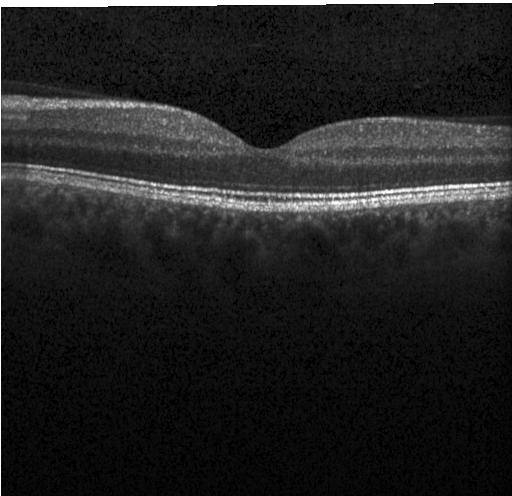
Impression: no evidence of CNV, DME, or drusen.